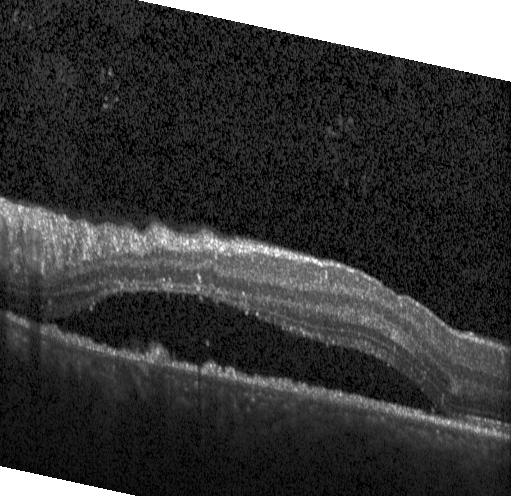 Macular OCT: choroidal neovascularization.